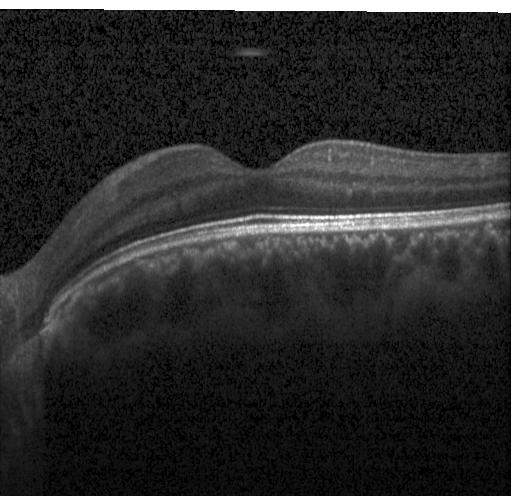

Optical coherence tomography B-scan; Heidelberg Spectralis OCT system — Diagnosis: neither choroidal neovascularization, diabetic macular edema, nor drusen.